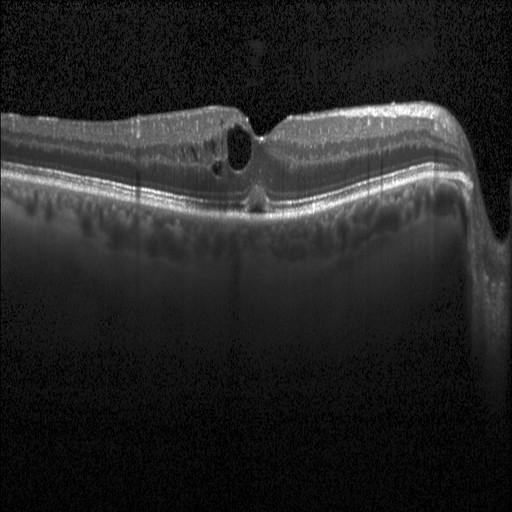
Through the macula, optical coherence tomography B-scan, Heidelberg Spectralis OCT system
Assessment: DME.